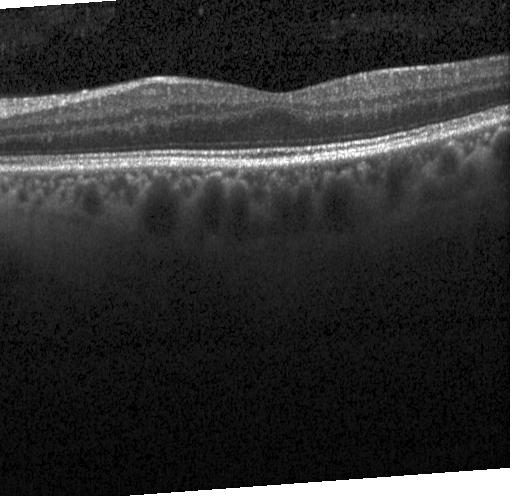
This B-scan demonstrates no choroidal neovascularization, diabetic macular edema, or drusen.